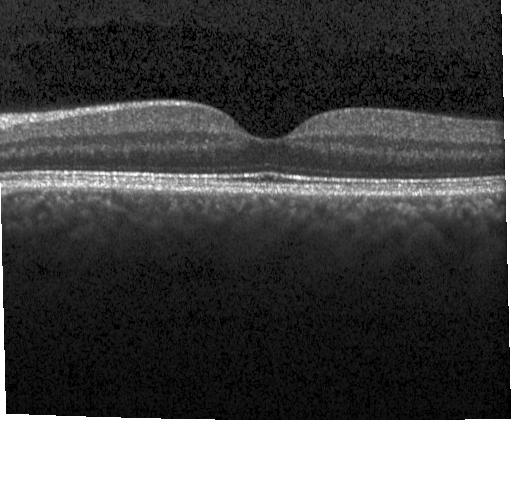
Retinal OCT cross-section; Heidelberg Spectralis OCT system; centered on the fovea
Impression: no CNV, DME, or drusen.